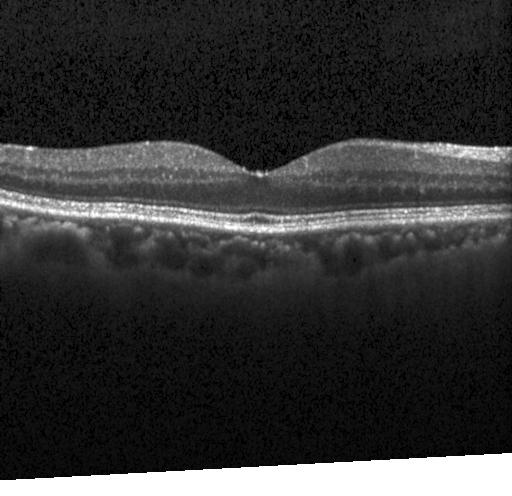
Impression: no CNV, DME, or drusen.